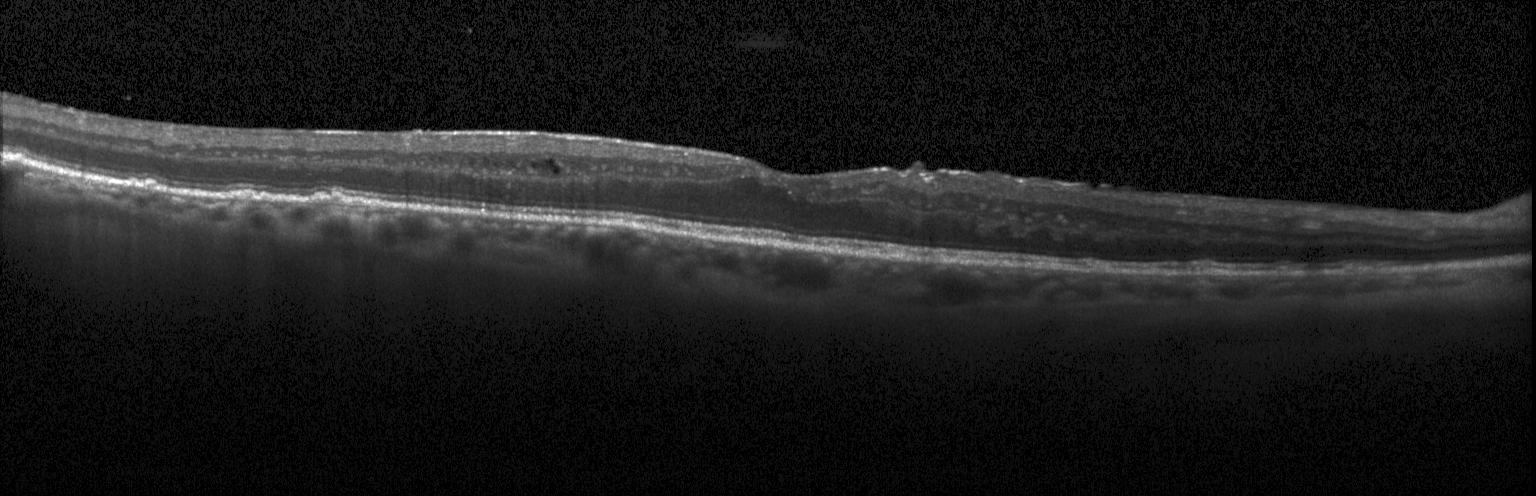

Retinal OCT cross-section; spectral-domain OCT.
Diabetic macular edema (DME).